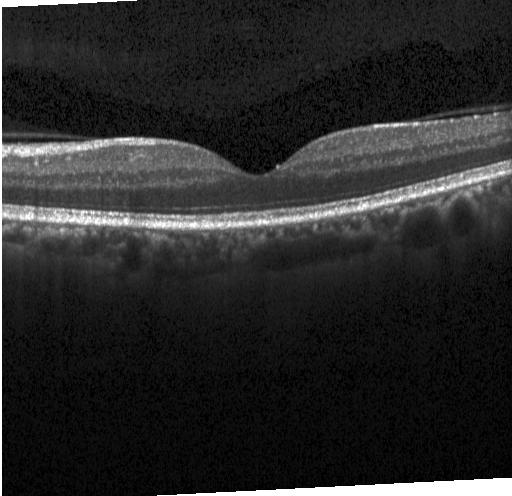 Impression: no CNV, DME, or drusen.